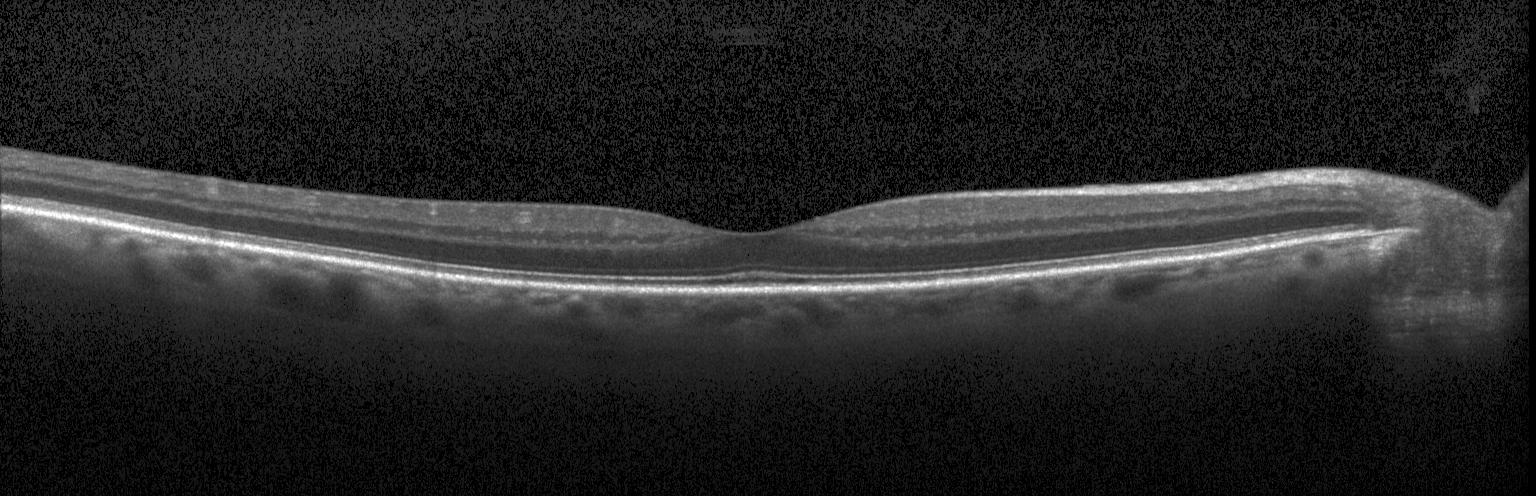

Retinal OCT B-scan.
The scan shows no evidence of choroidal neovascularization, diabetic macular edema, or drusen.